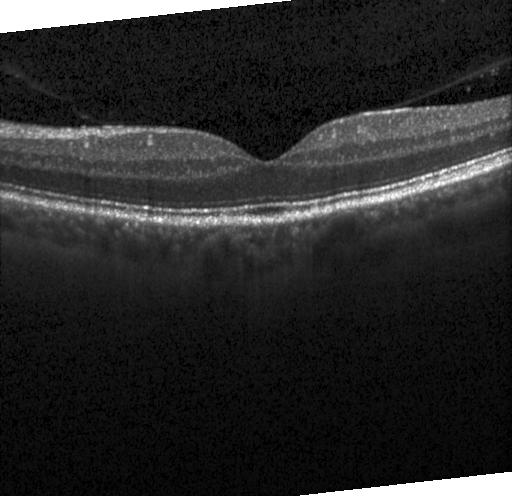

Dx: no CNV, DME, or drusen.